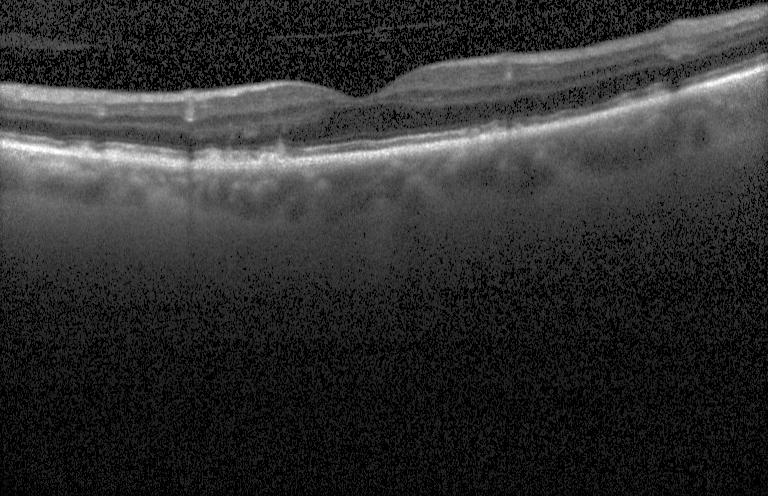

Spectral-domain optical coherence tomography; optical coherence tomography B-scan. OCT finding: multiple drusen.